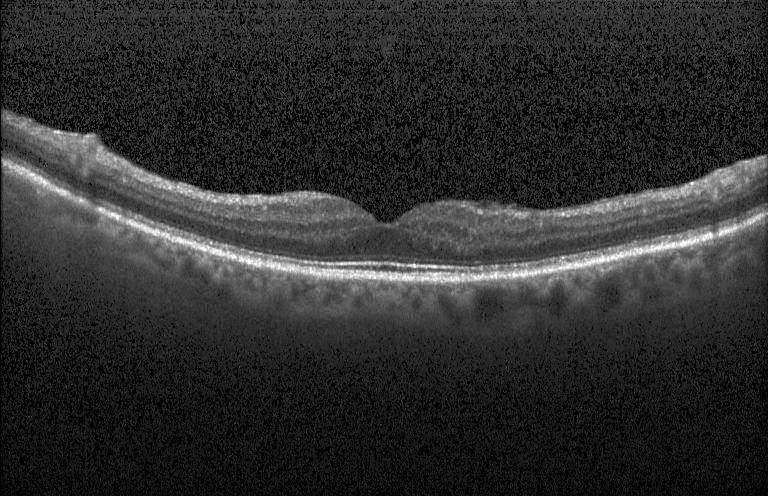 SD-OCT. Retinal OCT B-scan. Fovea-centered. Heidelberg Spectralis OCT system. Diagnosis: neither choroidal neovascularization, diabetic macular edema, nor drusen.